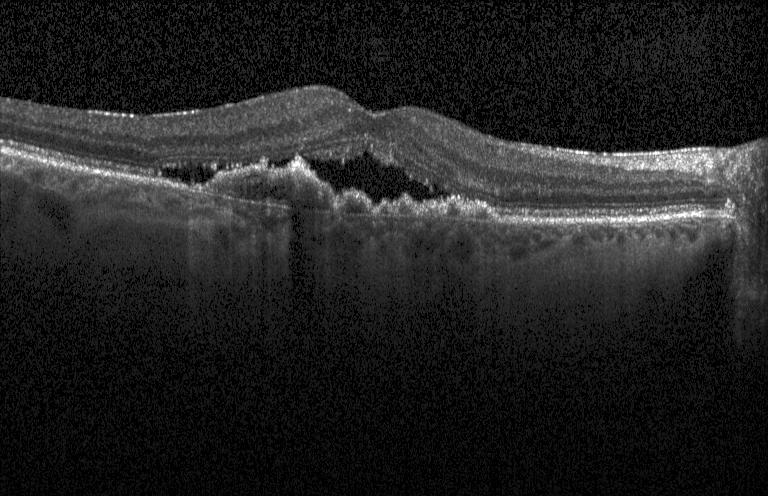

Optical coherence tomography B-scan.
Macular OCT: a choroidal neovascular membrane.